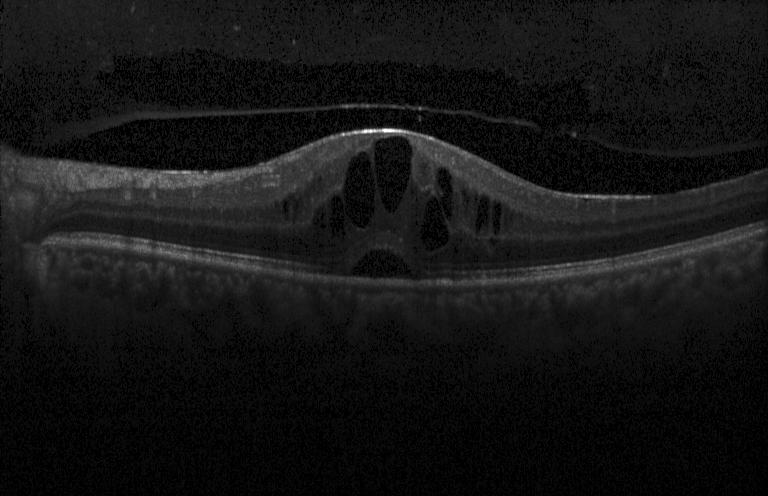 OCT finding: diabetic macular edema (DME).